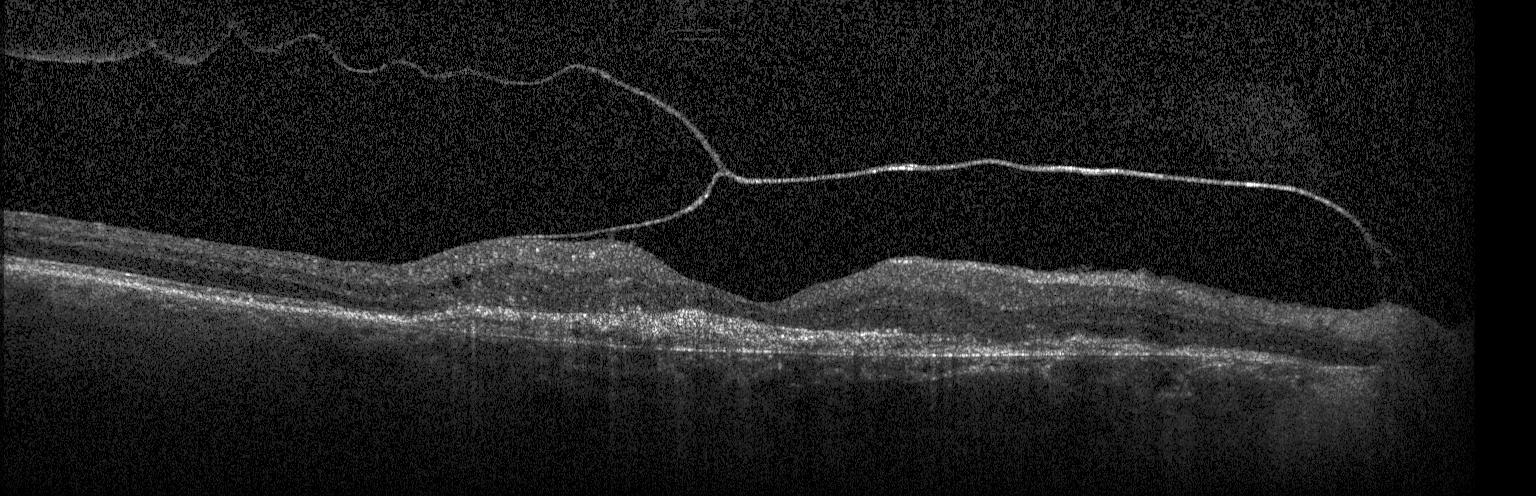 Spectral-domain optical coherence tomography, macular scan, optical coherence tomography scan.
Dx: a choroidal neovascular membrane.